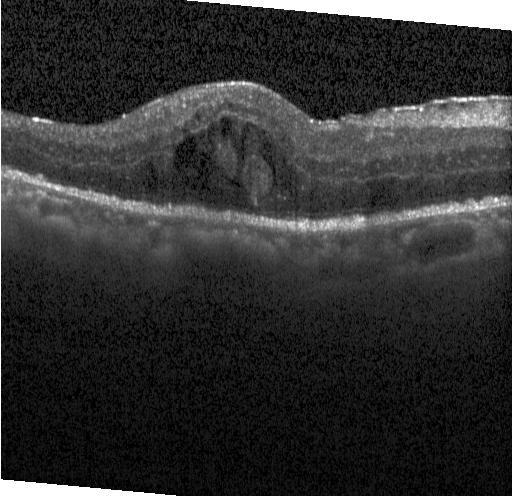
Dx: diabetic macular edema.